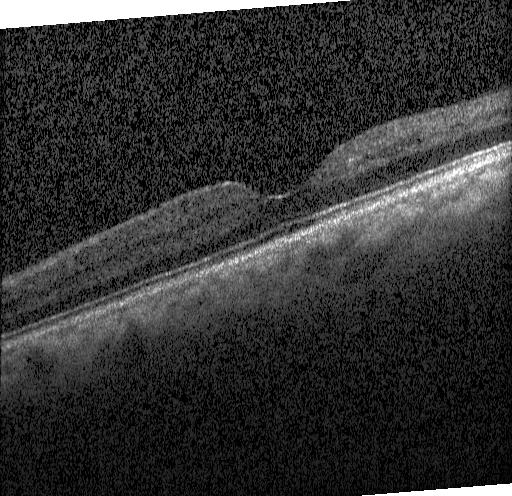 Spectral-domain optical coherence tomography. OCT line scan — Macular OCT: no evidence of choroidal neovascularization, diabetic macular edema, or drusen.